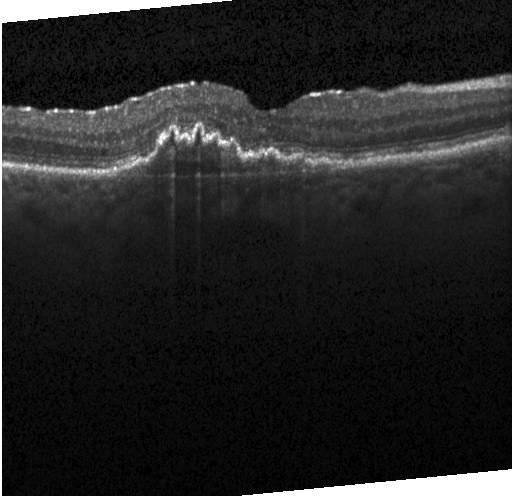
SD-OCT; instrument: Heidelberg Spectralis; retinal OCT cross-section; fovea-centered.
Finding: a choroidal neovascular membrane.